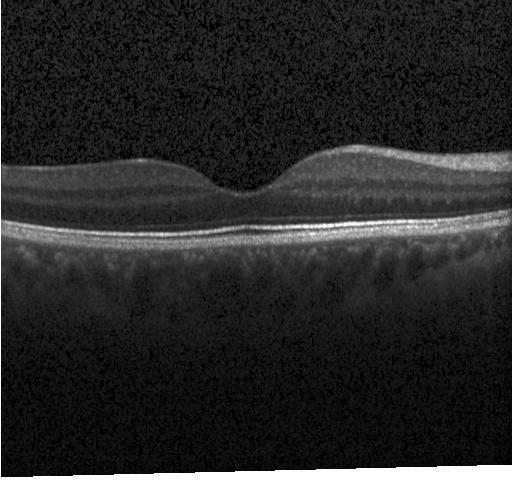 Through the macula, spectral-domain OCT, instrument: Heidelberg Spectralis, retinal OCT B-scan. Assessment: no evidence of choroidal neovascularization, diabetic macular edema, or drusen.